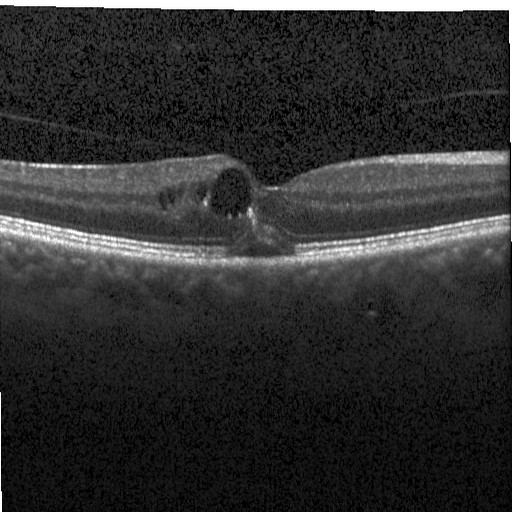

Optical coherence tomography scan · centered on the fovea
This B-scan demonstrates diabetic macular edema.